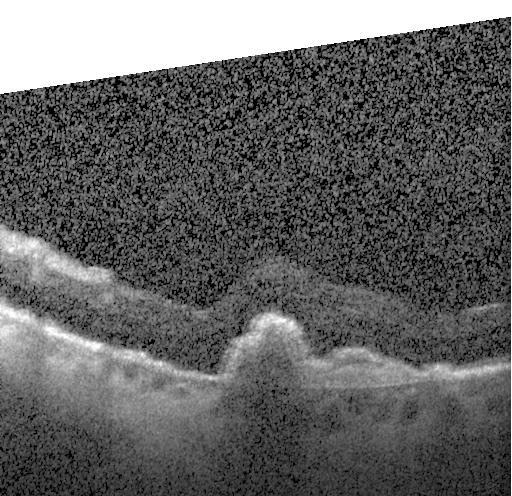
This B-scan demonstrates CNV.